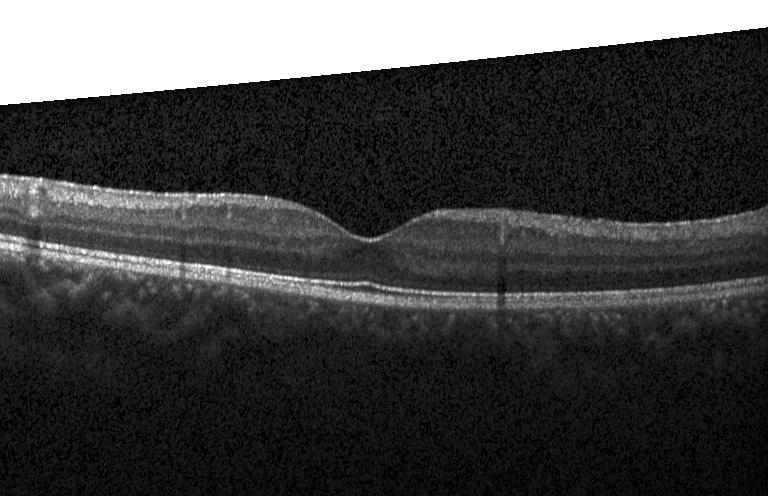

OCT finding: no CNV, no DME, and no drusen.